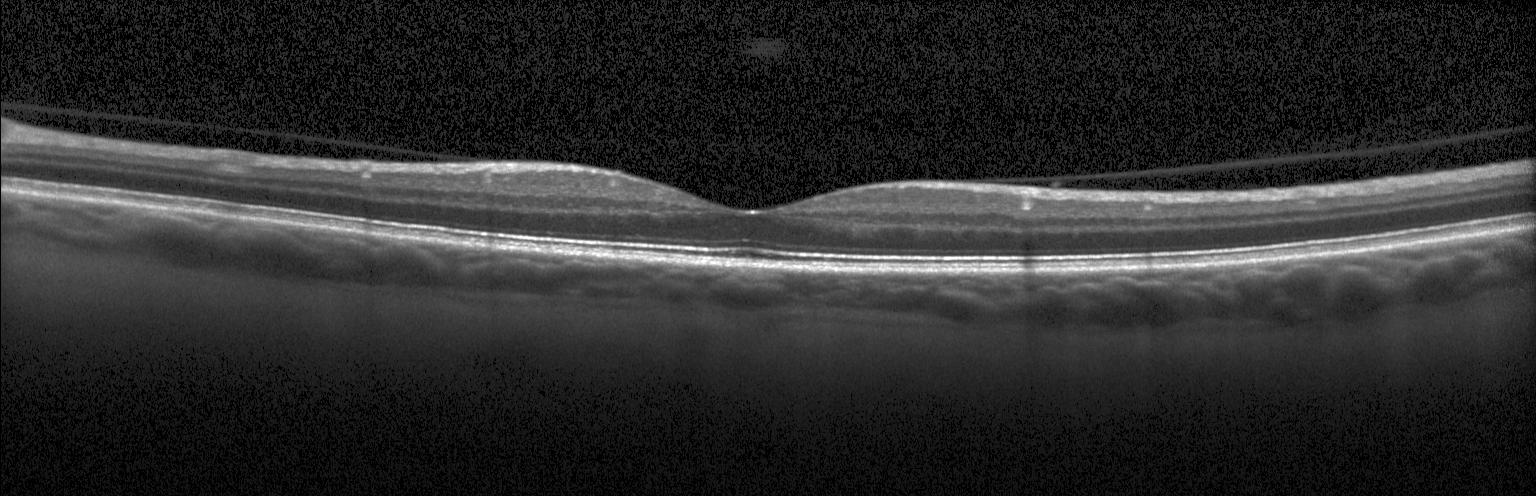

Finding: neither choroidal neovascularization, diabetic macular edema, nor drusen.